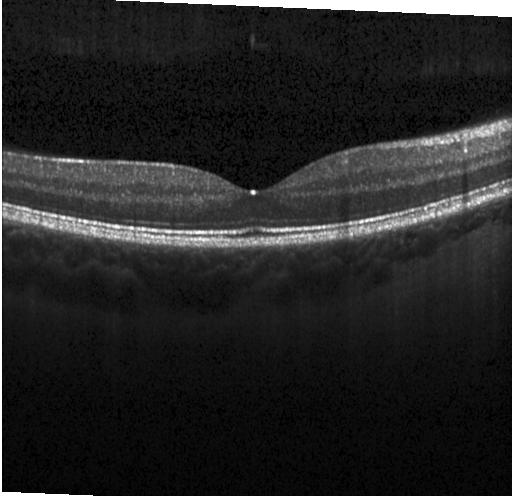

Finding: neither choroidal neovascularization, diabetic macular edema, nor drusen.